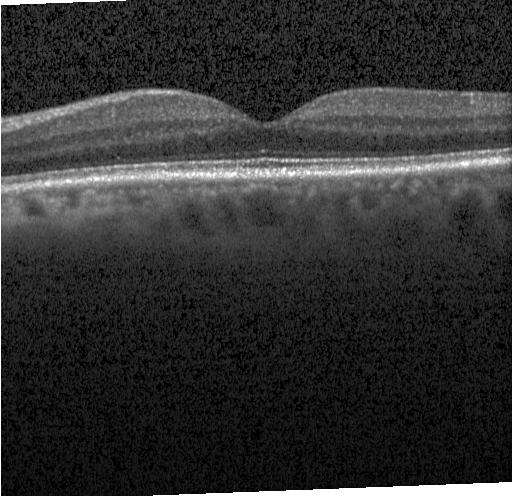 Finding: neither choroidal neovascularization, diabetic macular edema, nor drusen.